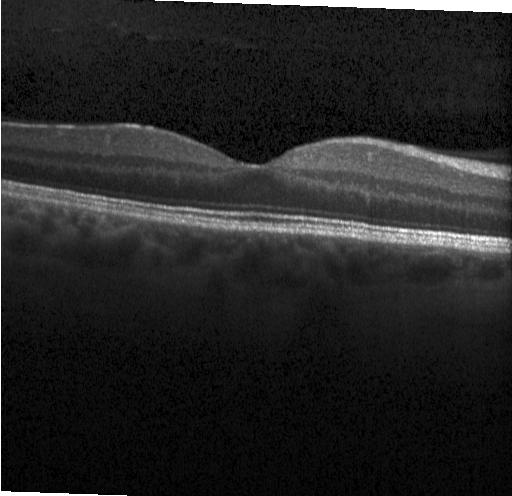 OCT B-scan — Impression: no evidence of choroidal neovascularization, diabetic macular edema, or drusen.